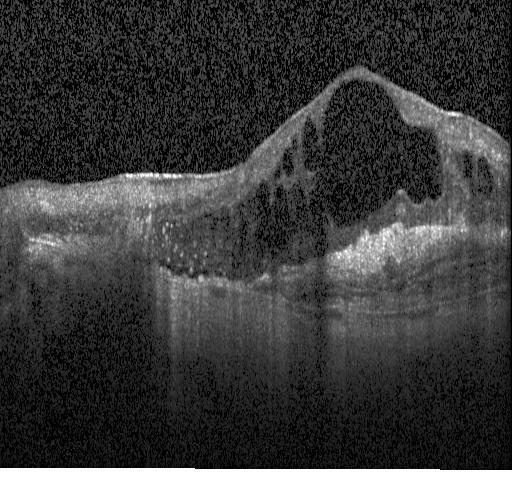
Spectral-domain OCT B-scan: choroidal neovascularization.